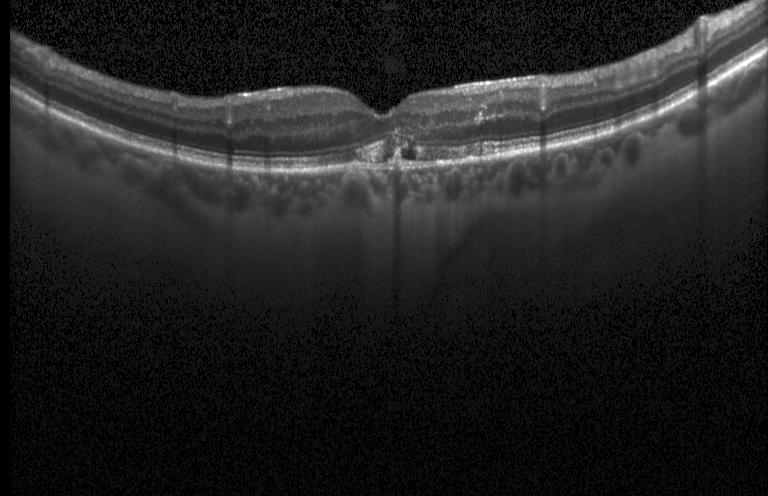

Through the macula; Heidelberg Spectralis OCT system; spectral-domain optical coherence tomography; retinal OCT cross-section.
A choroidal neovascular membrane.